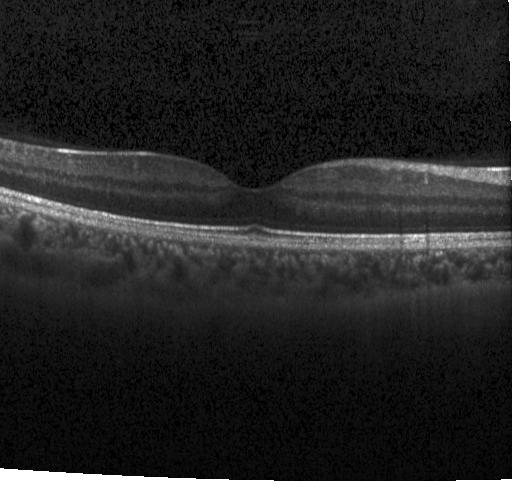
The scan shows no CNV, no DME, and no drusen.